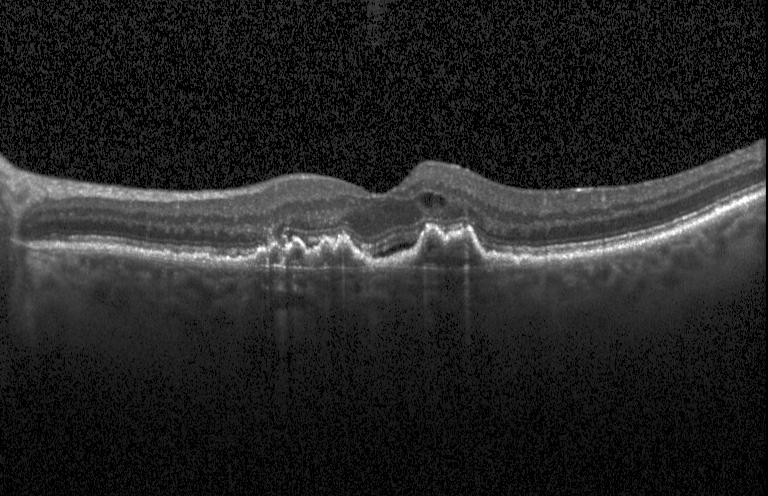
The scan shows CNV.